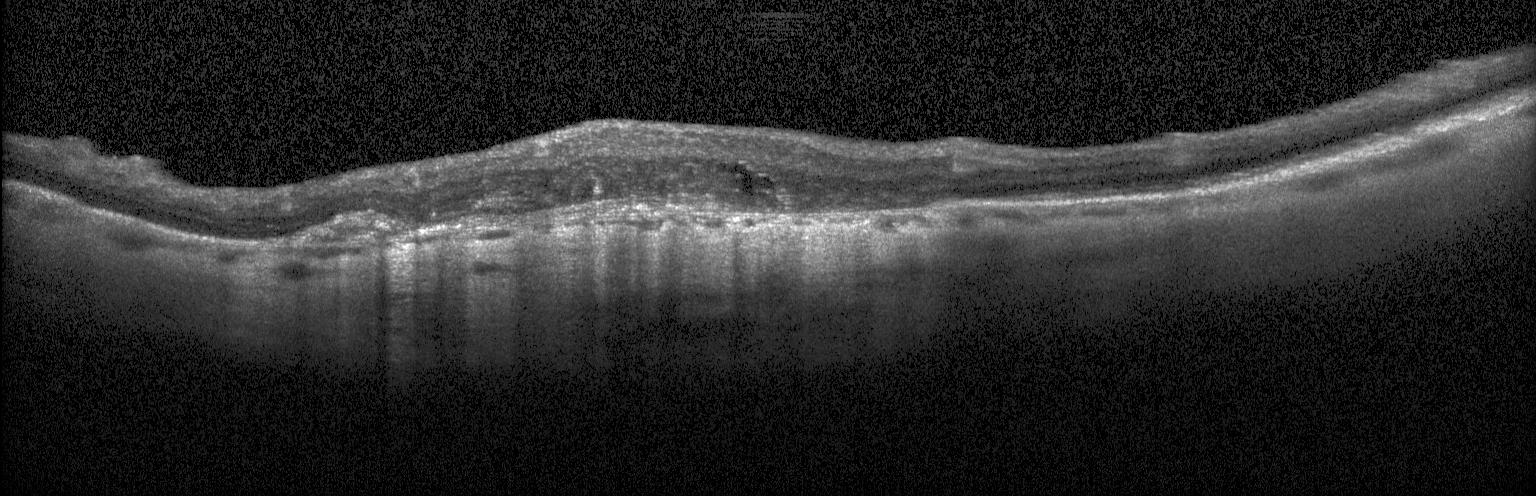
OCT B-scan. OCT finding: a choroidal neovascular membrane.